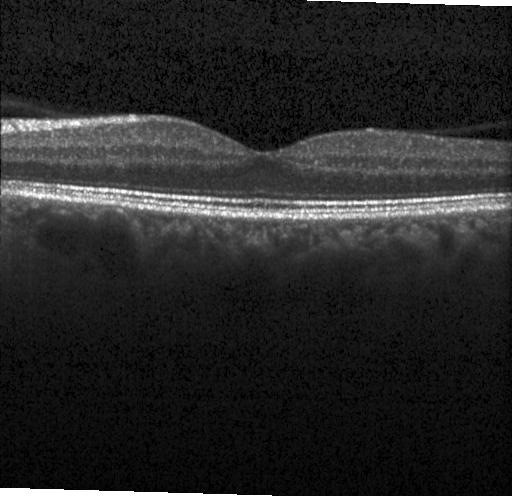

Diagnosis: neither CNV, DME, nor drusen.